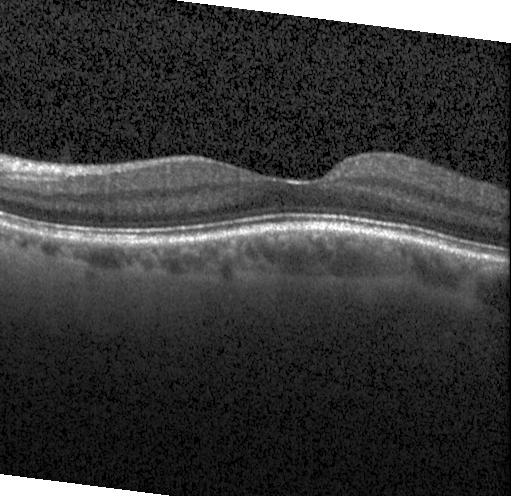
Dx: no evidence of choroidal neovascularization, diabetic macular edema, or drusen.